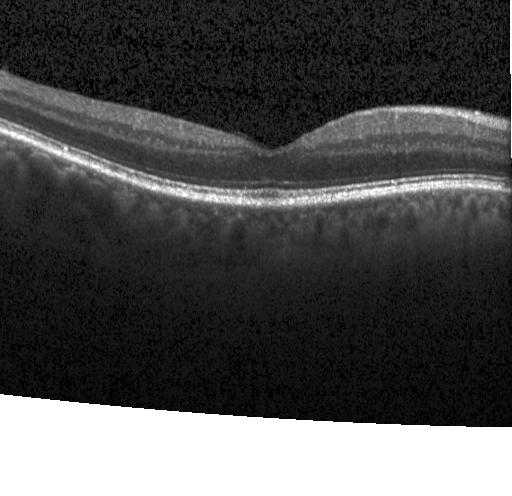

Retinal OCT cross-section showing no CNV, no DME, and no drusen.